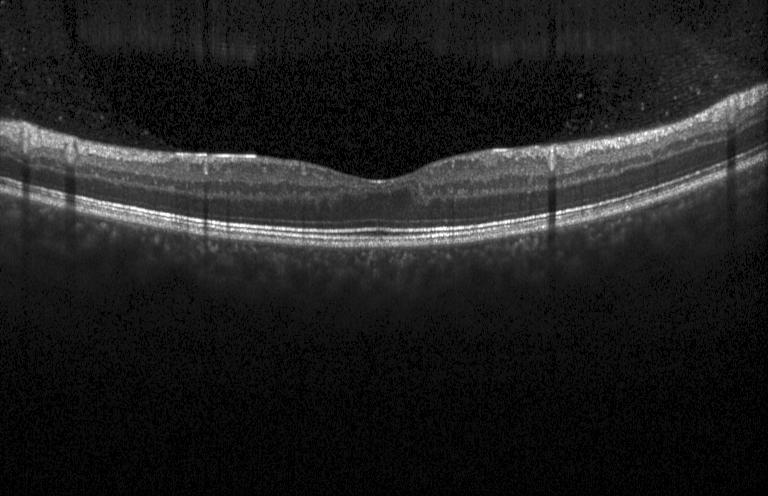

Assessment: no choroidal neovascularization, no diabetic macular edema, and no drusen.